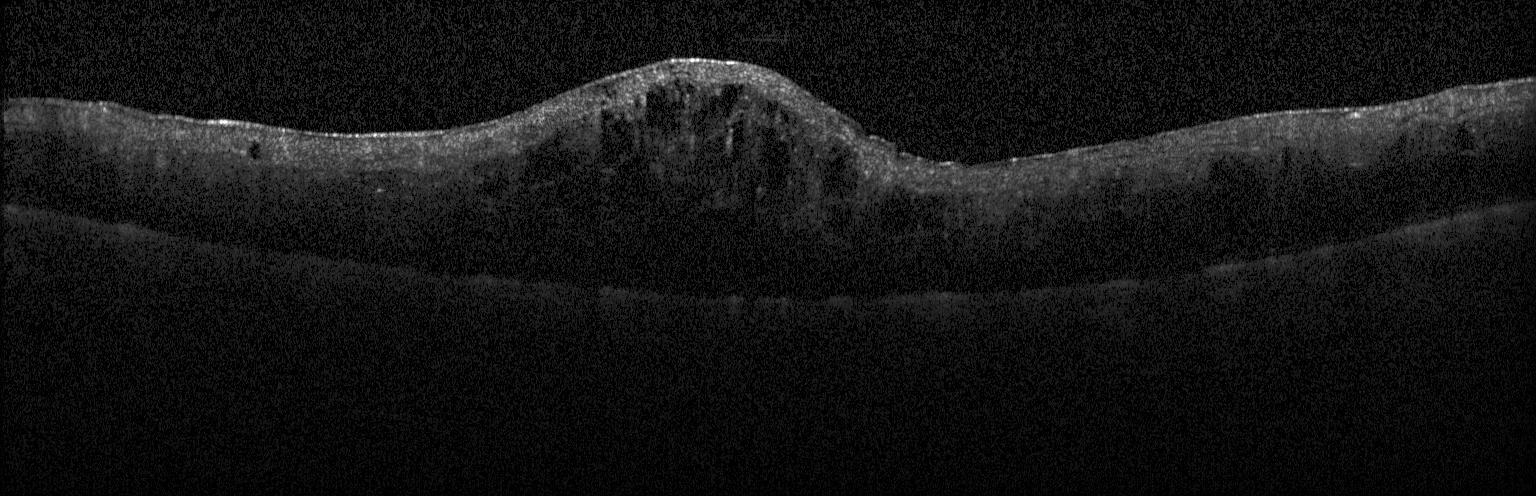

OCT B-scan · instrument: Heidelberg Spectralis · fovea-centered · SD-OCT. Finding: DME.